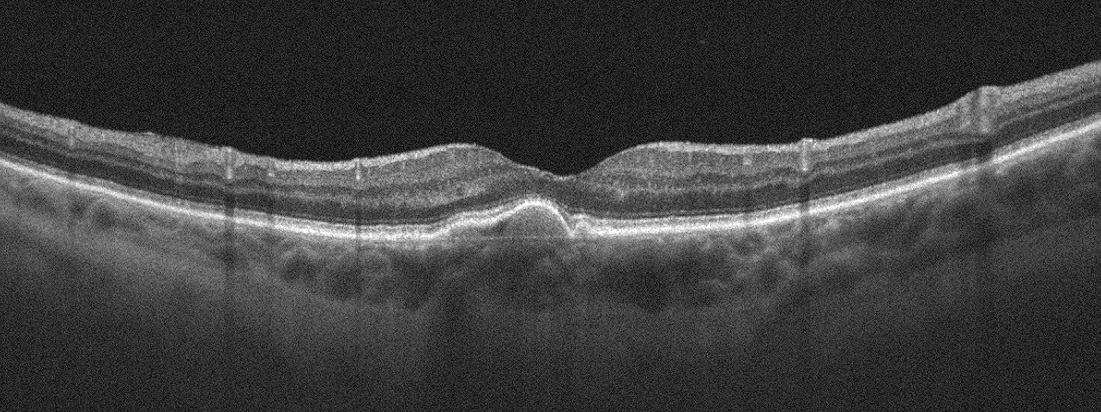
OCT line scan
The scan shows age-related macular degeneration (AMD).